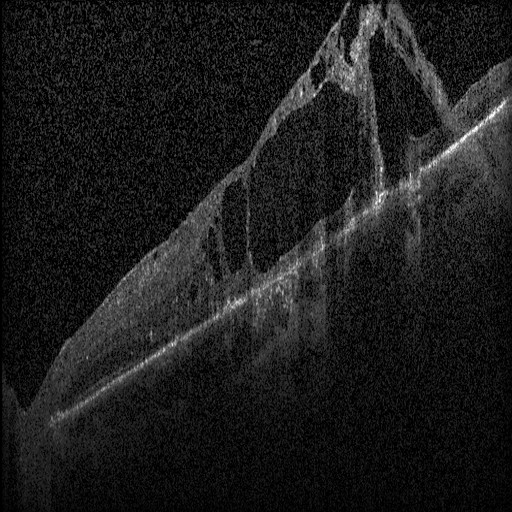
Finding: diabetic macular edema.